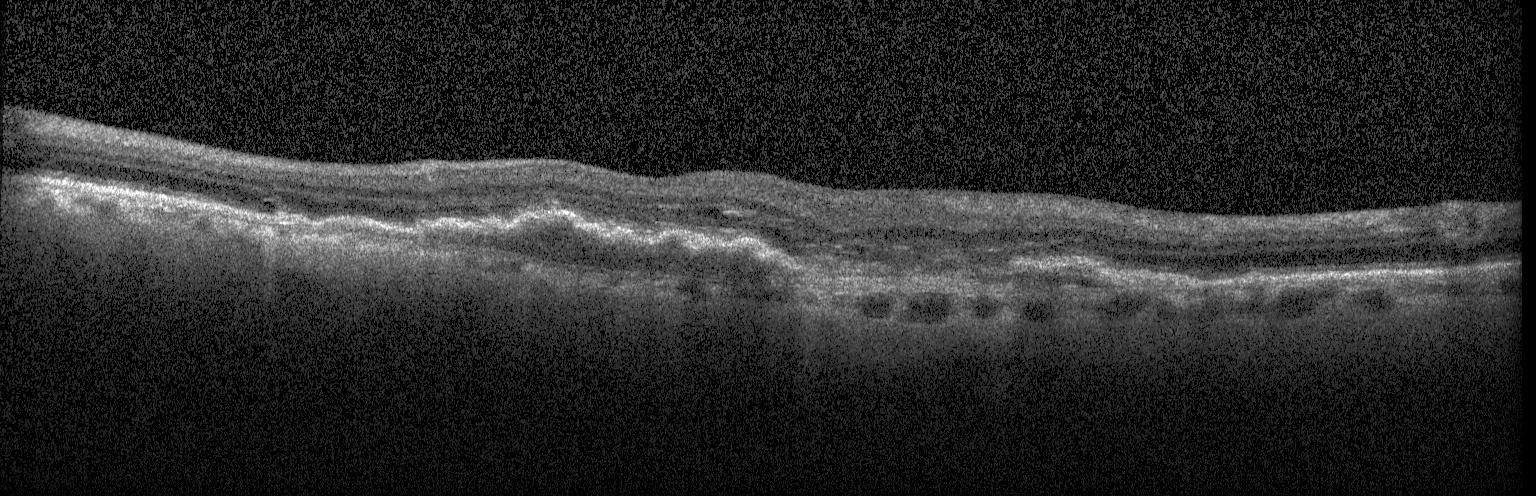
Assessment: a choroidal neovascular membrane.